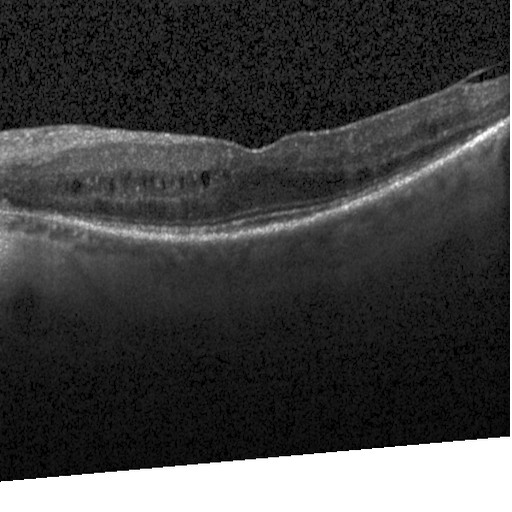 Optical coherence tomography B-scan. DME.